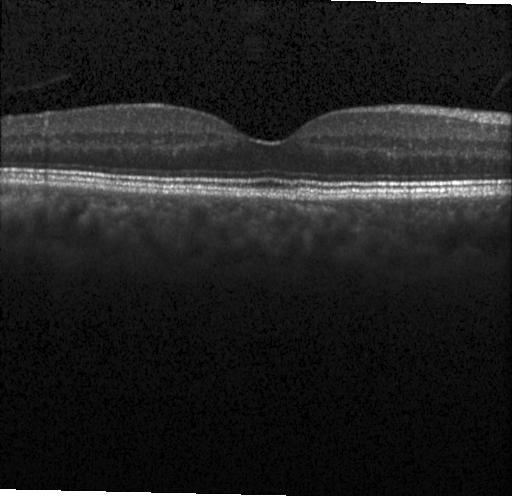

OCT line scan
Macular OCT: no CNV, no DME, and no drusen.